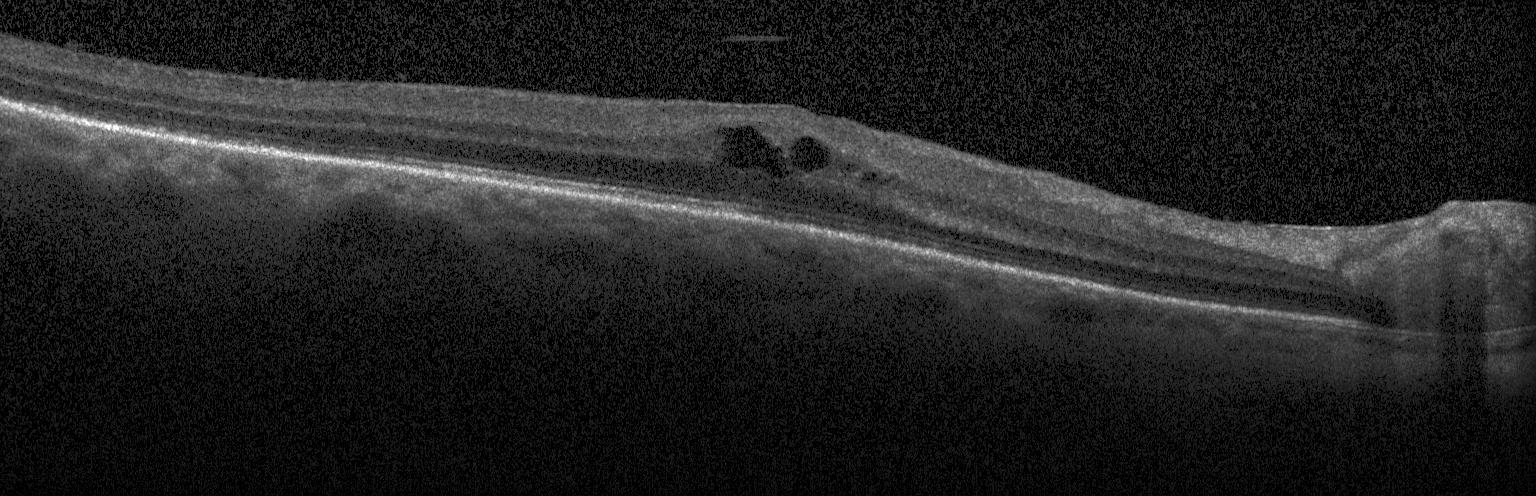
Retinal OCT cross-section. DME.